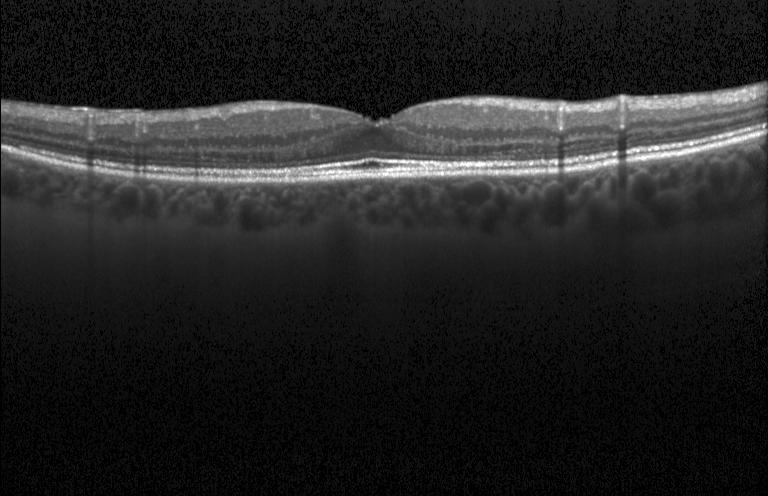 Assessment: no CNV, DME, or drusen.